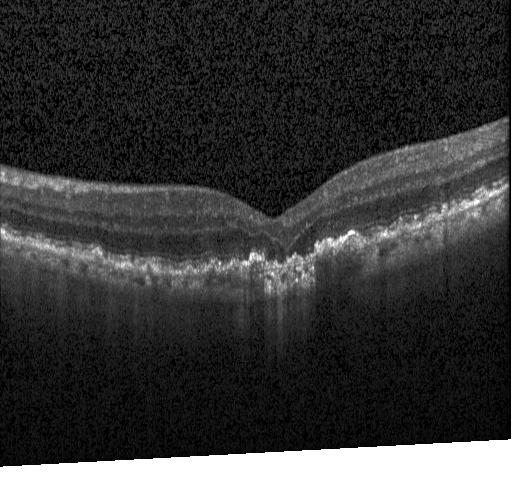 Macular scan, acquired on a Heidelberg Spectralis, OCT B-scan, spectral-domain OCT
Finding: choroidal neovascularization (CNV).